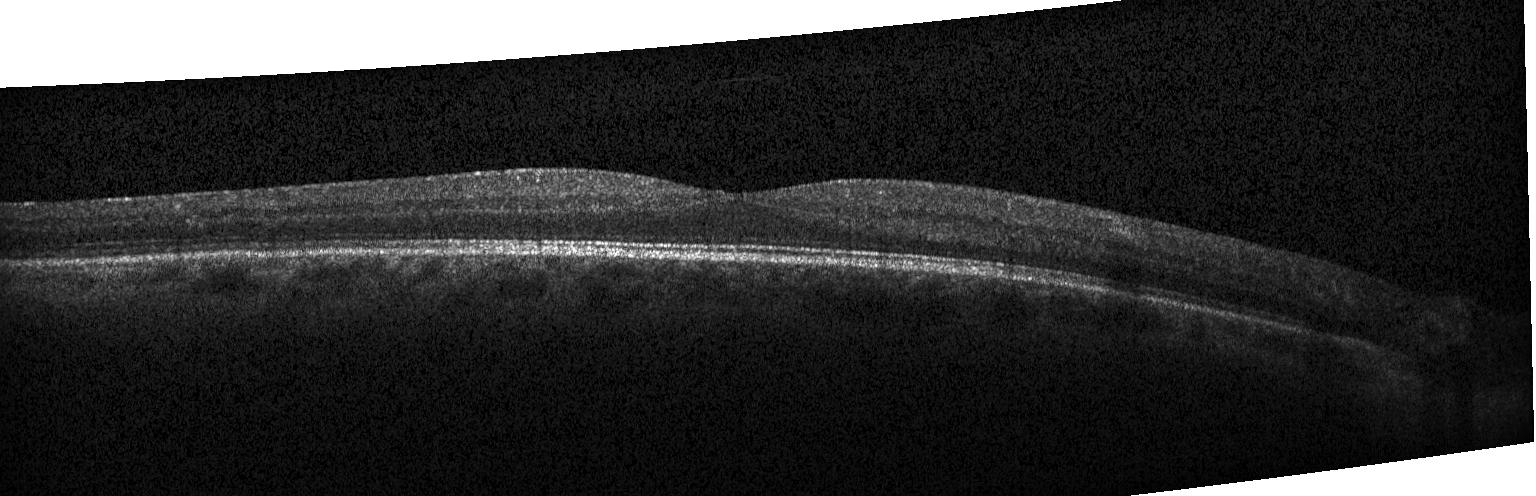
Spectral-domain OCT; optical coherence tomography B-scan; Heidelberg Spectralis OCT system
Diagnosis: no choroidal neovascularization, diabetic macular edema, or drusen.